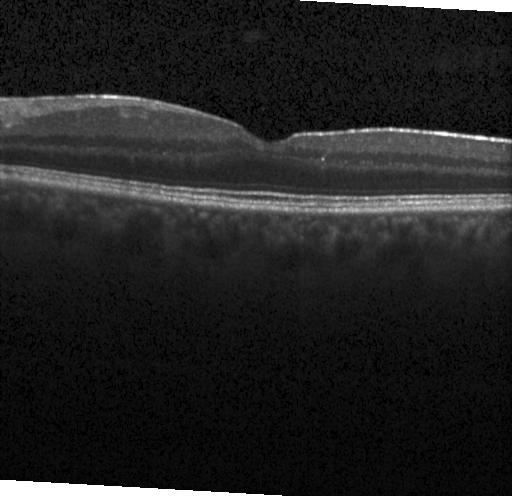

Macular scan; spectral-domain OCT; optical coherence tomography scan; instrument: Heidelberg Spectralis.
Neither CNV, DME, nor drusen.